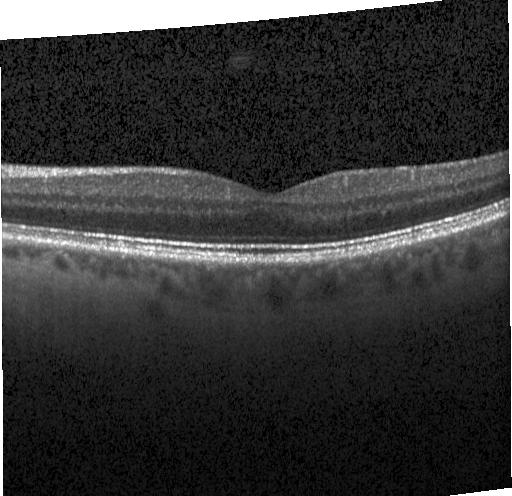

Macular OCT: no choroidal neovascularization, no diabetic macular edema, and no drusen.